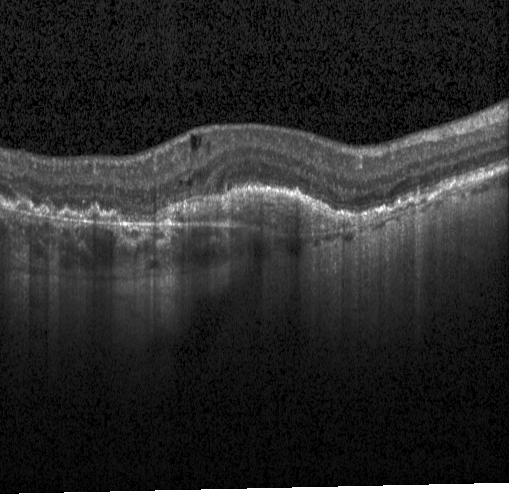
Macular scan, OCT B-scan, SD-OCT.
Finding: choroidal neovascularization.